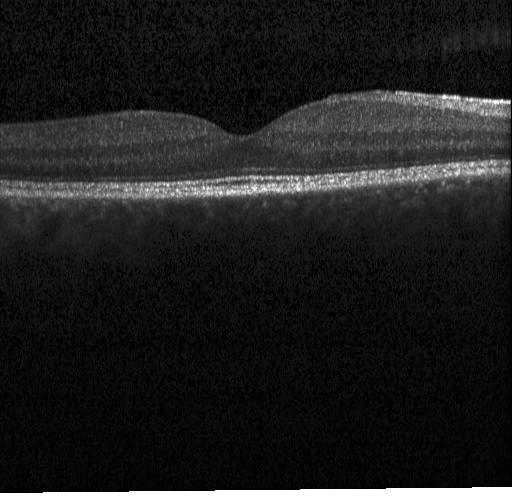 Macular scan. Retinal OCT cross-section — Finding: no CNV, DME, or drusen.